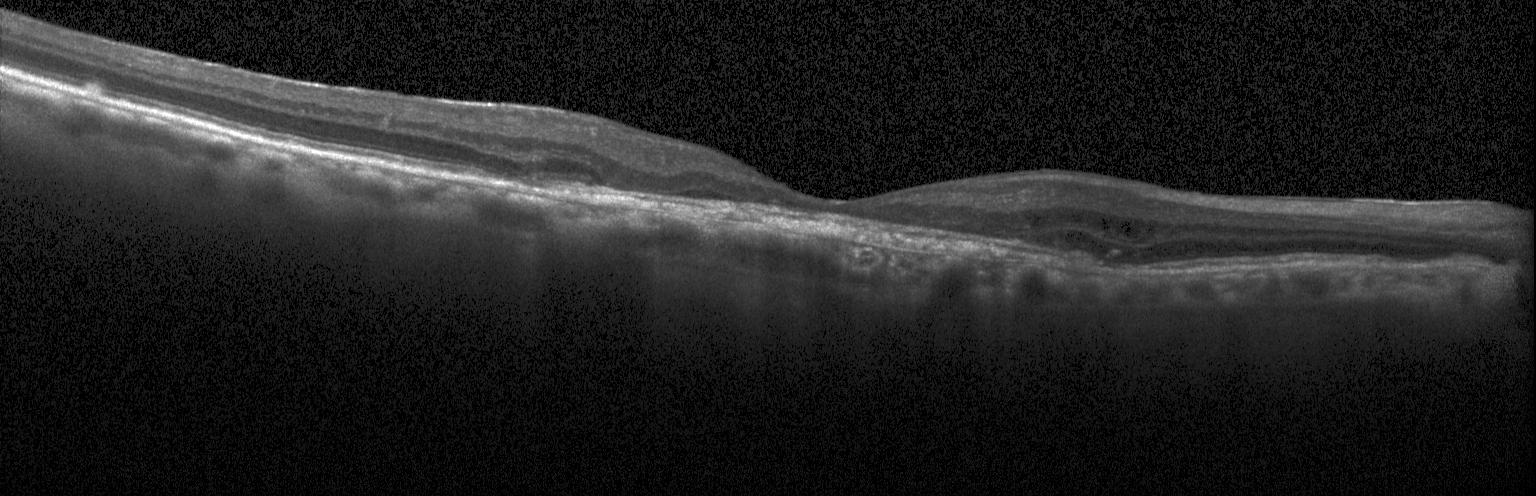
Instrument: Heidelberg Spectralis, SD-OCT, retinal OCT B-scan, fovea-centered. Finding: CNV.